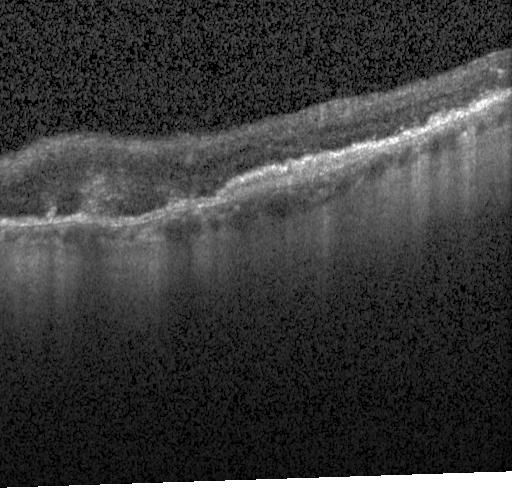
Diagnosis: a choroidal neovascular membrane.